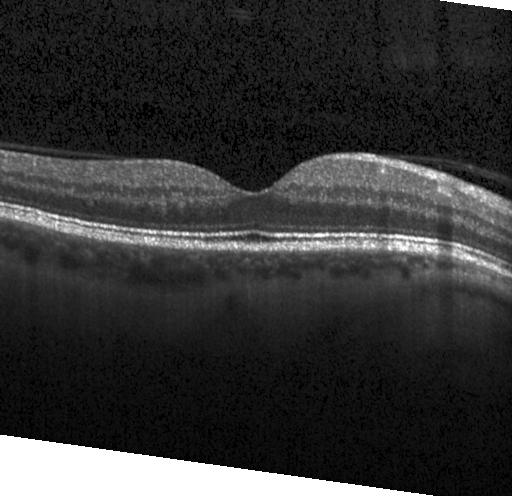 OCT line scan. Through the macula — OCT finding: neither CNV, DME, nor drusen.